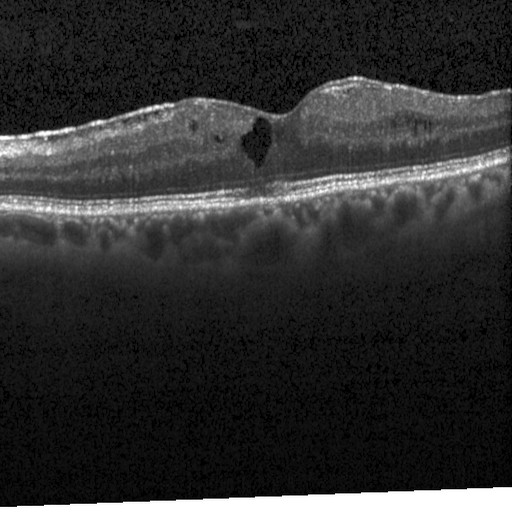
OCT B-scan.
Finding: diabetic macular edema.